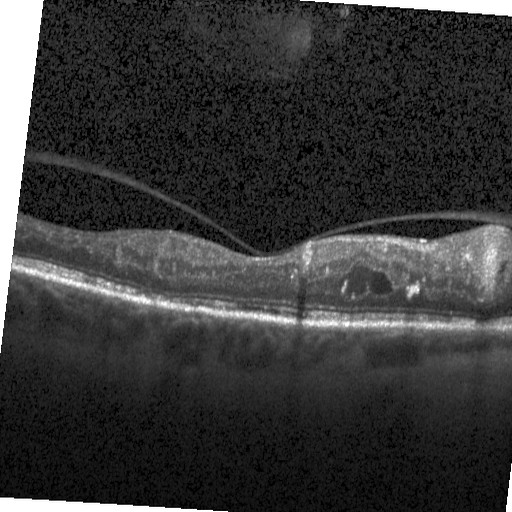 Retinal OCT B-scan · spectral-domain OCT. Diagnosis: diabetic macular edema.